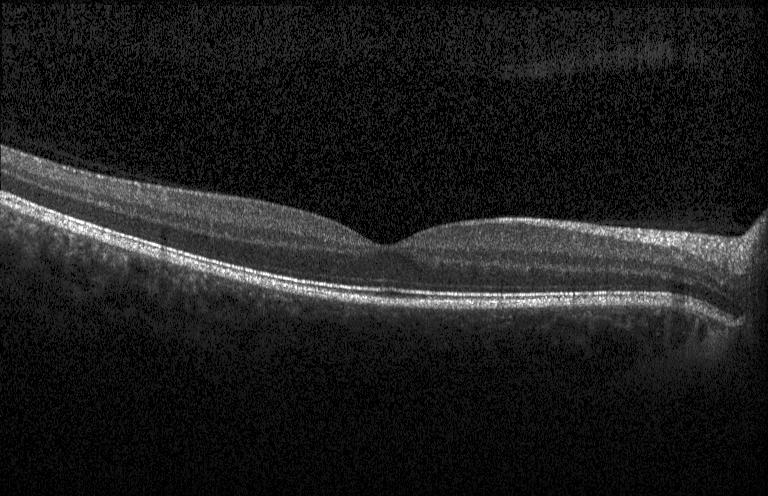
Optical coherence tomography scan; horizontal scan through the fovea — Diagnosis: no choroidal neovascularization, no diabetic macular edema, and no drusen.